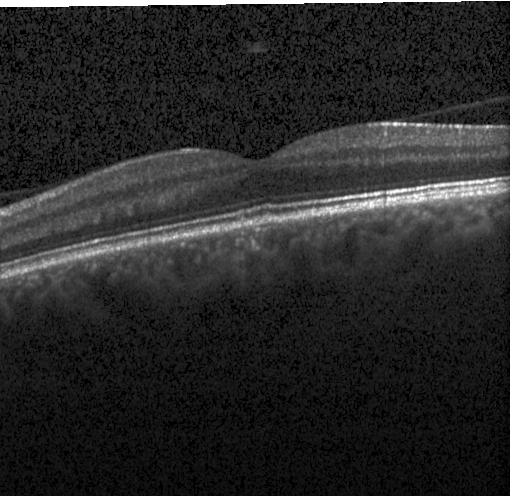

Horizontal scan through the fovea · OCT B-scan · SD-OCT · Heidelberg Spectralis
Finding: no choroidal neovascularization, diabetic macular edema, or drusen.